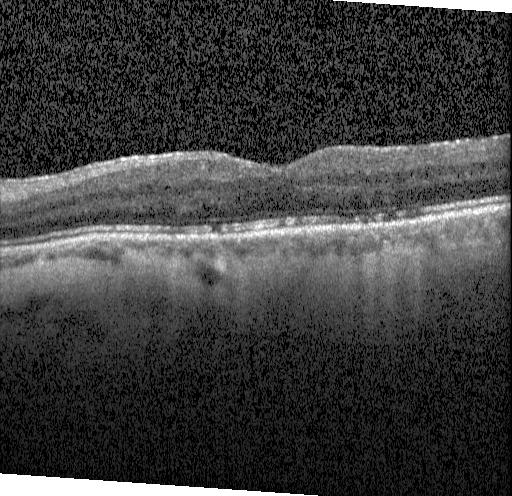 Centered on the fovea. Retinal OCT B-scan. SD-OCT. Heidelberg Spectralis. Diagnosis: neither CNV, DME, nor drusen.